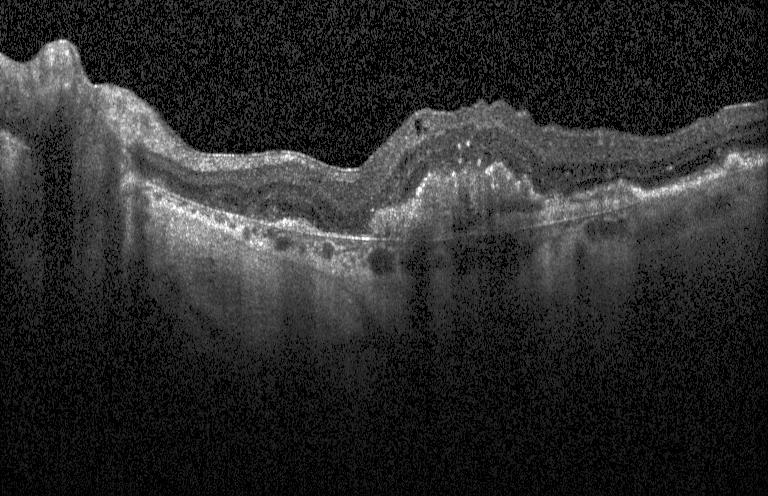

Spectral-domain OCT B-scan: a choroidal neovascular membrane.